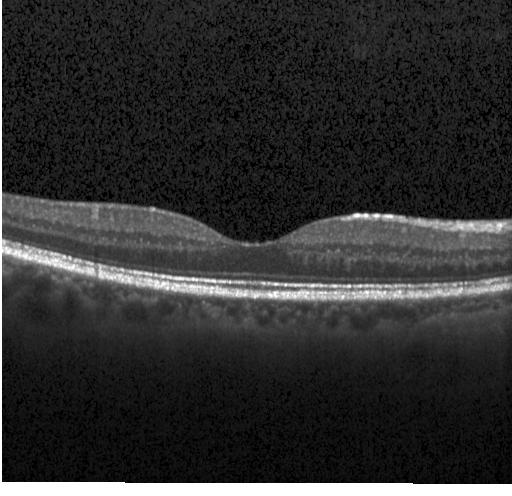

Assessment: no choroidal neovascularization, no diabetic macular edema, and no drusen.